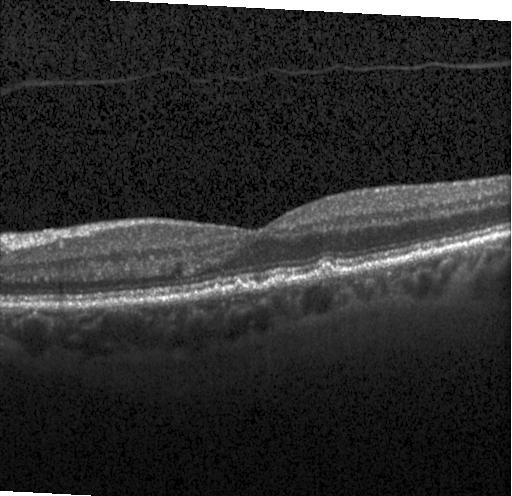

Macular OCT: drusen.